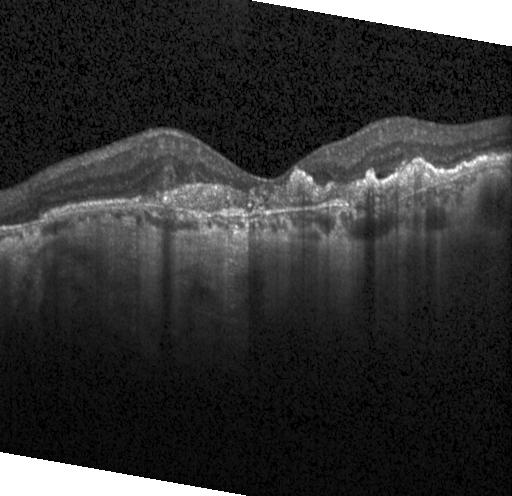
Retinal OCT B-scan — Impression: choroidal neovascularization (CNV).